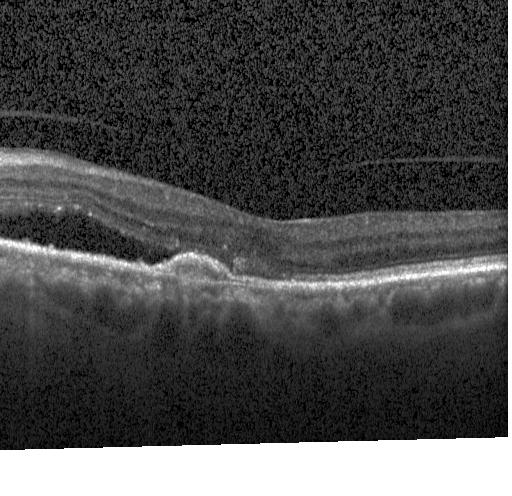
OCT B-scan.
Dx: a choroidal neovascular membrane.